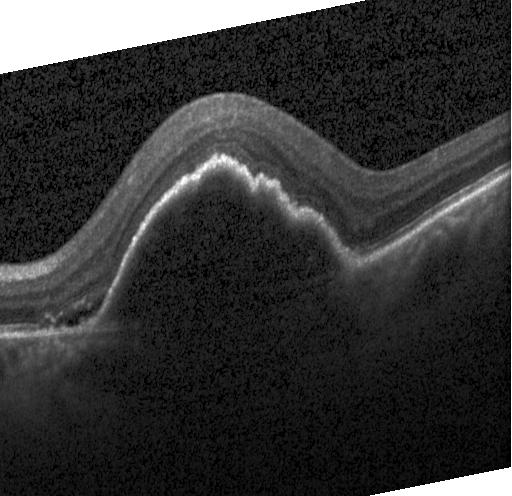

Optical coherence tomography scan
Finding: choroidal neovascularization (CNV).